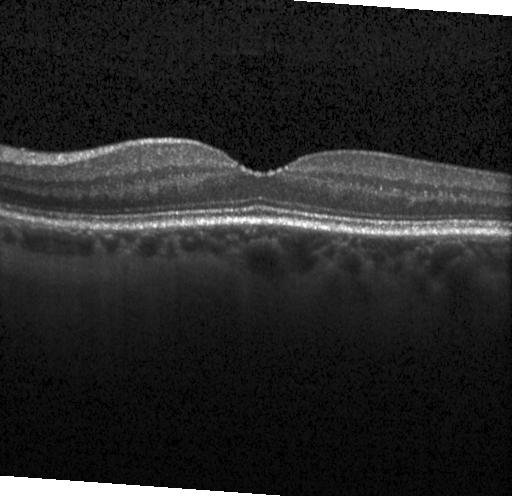

This B-scan demonstrates no CNV, DME, or drusen.